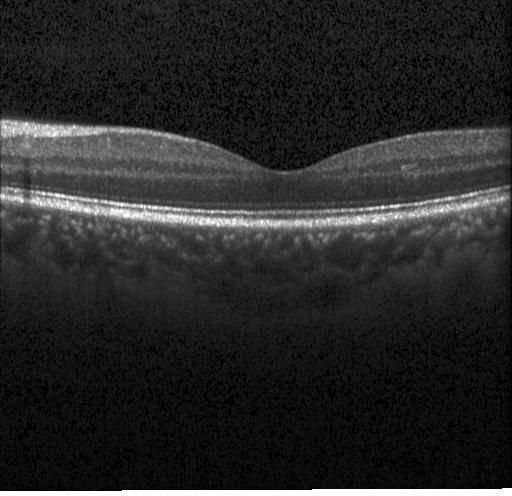
OCT B-scan
Macular OCT: no choroidal neovascularization, no diabetic macular edema, and no drusen.